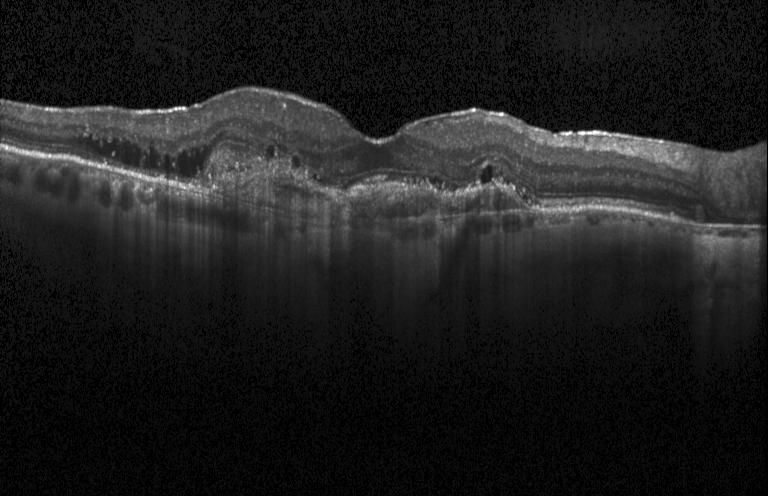

Instrument: Heidelberg Spectralis · optical coherence tomography scan · spectral-domain OCT
Diagnosis: a choroidal neovascular membrane.